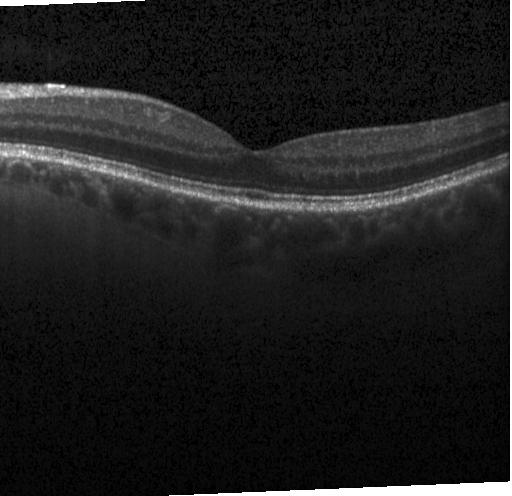
Retinal OCT cross-section showing no choroidal neovascularization, no diabetic macular edema, and no drusen.